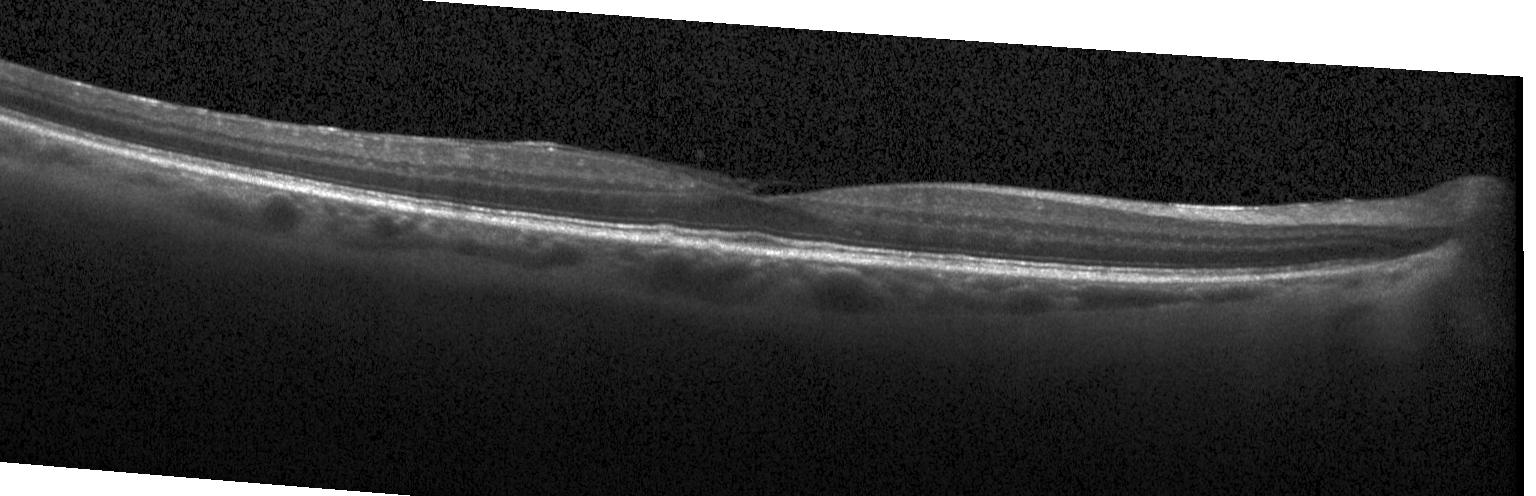
The scan shows multiple drusen.